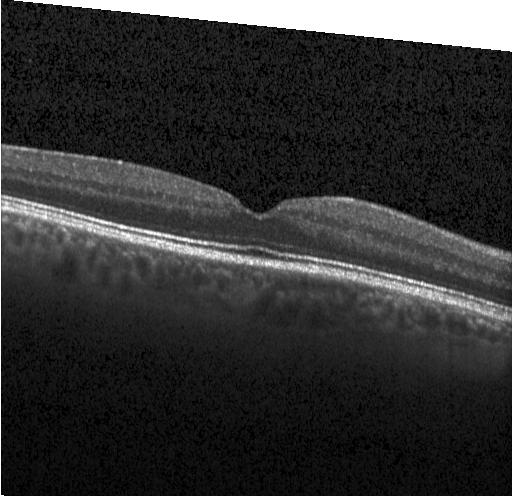 Macular scan; OCT line scan; SD-OCT; instrument: Heidelberg Spectralis
Assessment: no choroidal neovascularization, no diabetic macular edema, and no drusen.